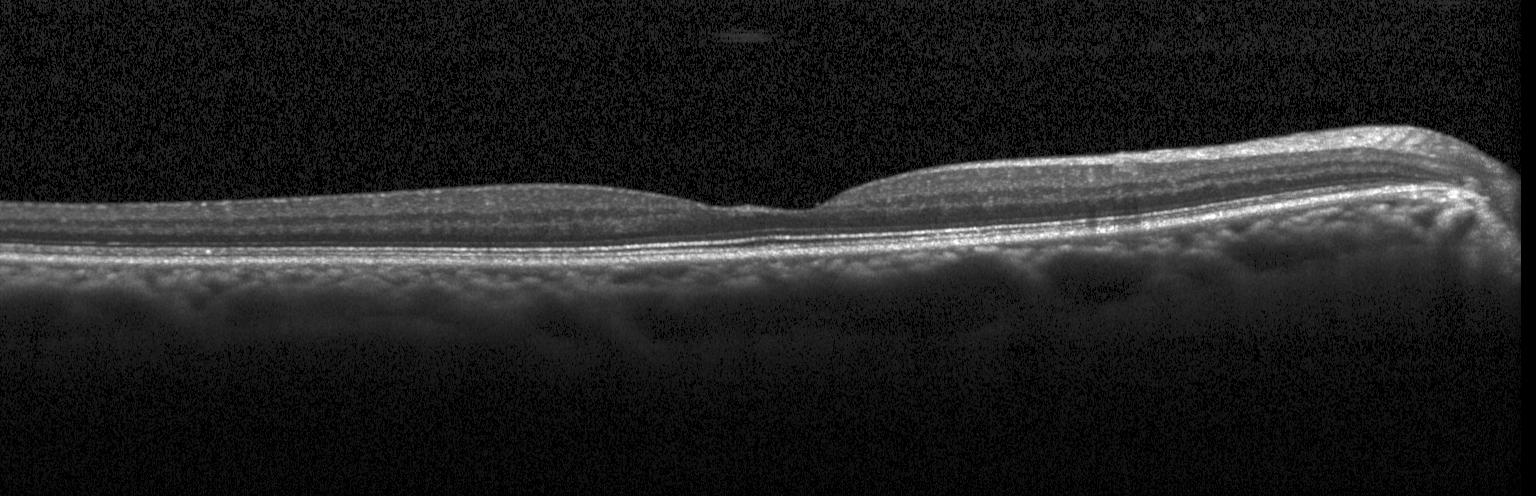

Dx: no choroidal neovascularization, diabetic macular edema, or drusen.